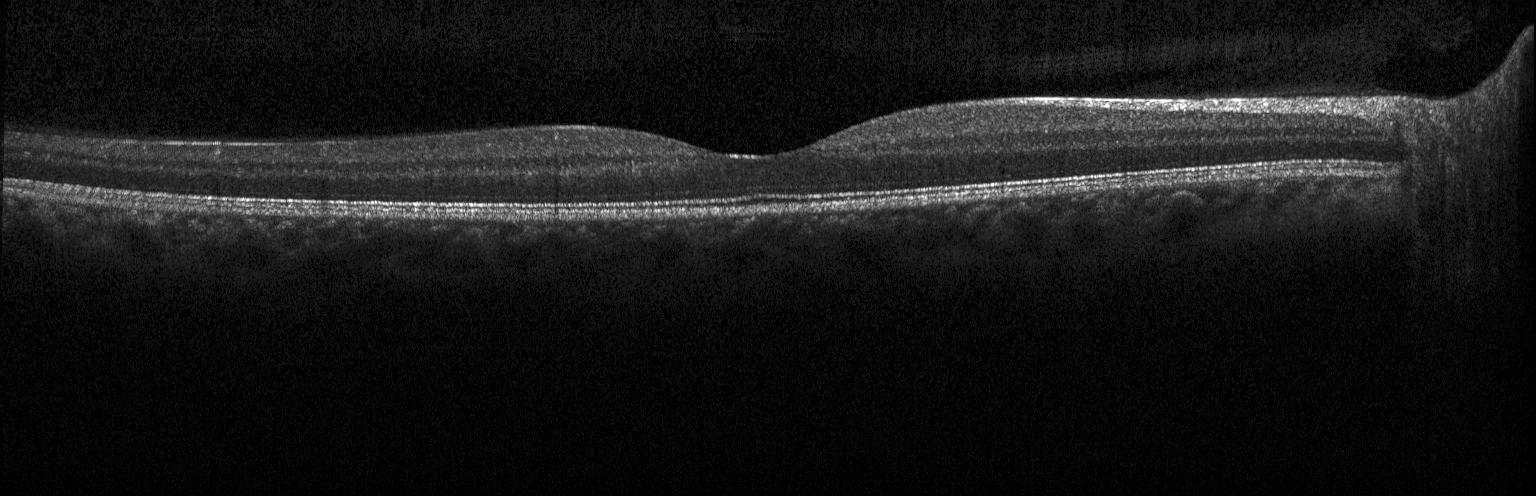 Heidelberg Spectralis. Retinal OCT B-scan. Fovea-centered
Finding: neither CNV, DME, nor drusen.